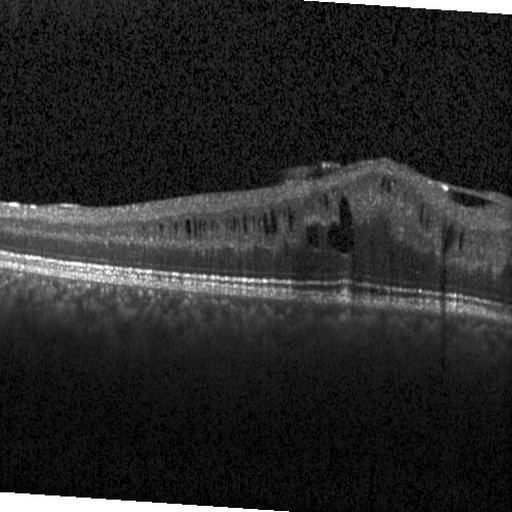

Diagnosis: diabetic macular edema (DME).